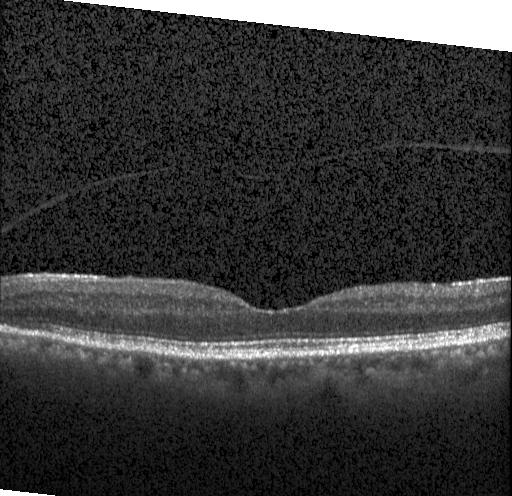 OCT B-scan; Heidelberg Spectralis OCT system; spectral-domain OCT — Impression: no choroidal neovascularization, diabetic macular edema, or drusen.